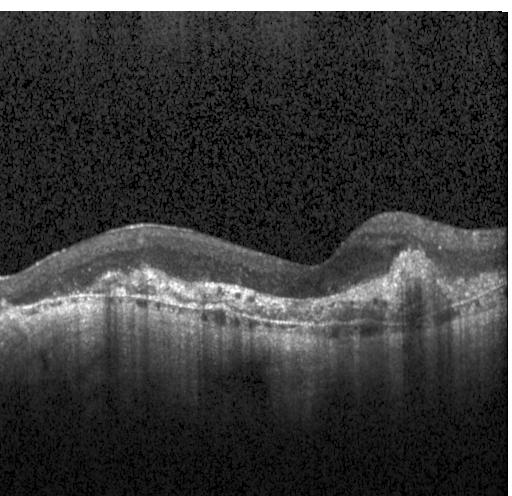

Macular OCT: a choroidal neovascular membrane.